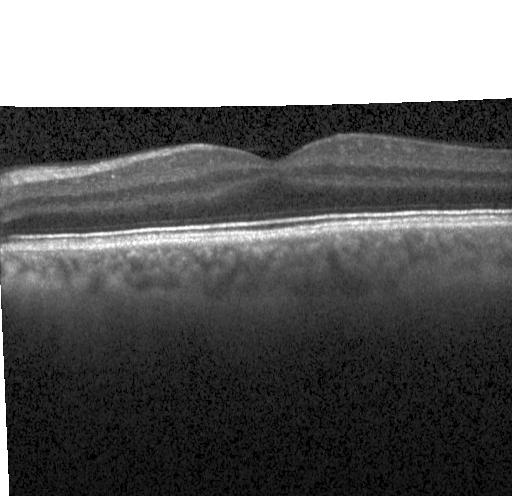
SD-OCT · optical coherence tomography scan · instrument: Heidelberg Spectralis · fovea-centered.
Macular OCT: neither choroidal neovascularization, diabetic macular edema, nor drusen.